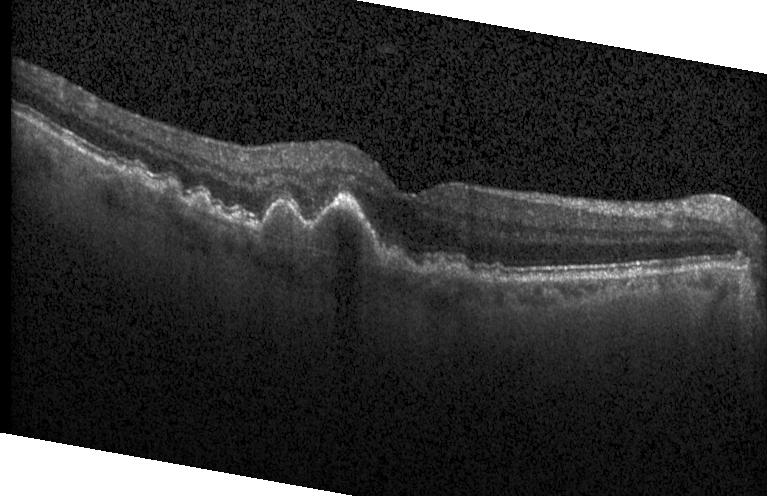

Retinal OCT B-scan
Impression: CNV.